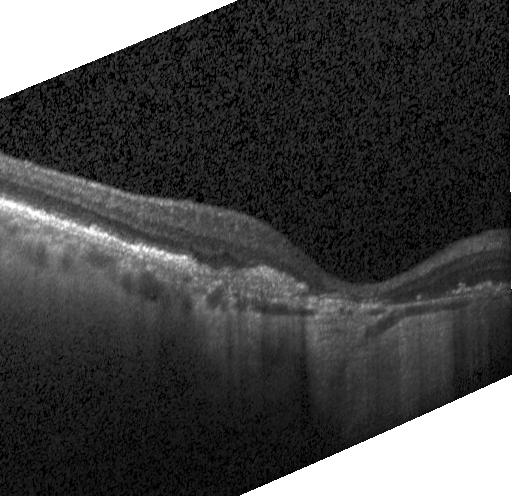

Instrument: Heidelberg Spectralis, OCT line scan — Dx: a choroidal neovascular membrane.